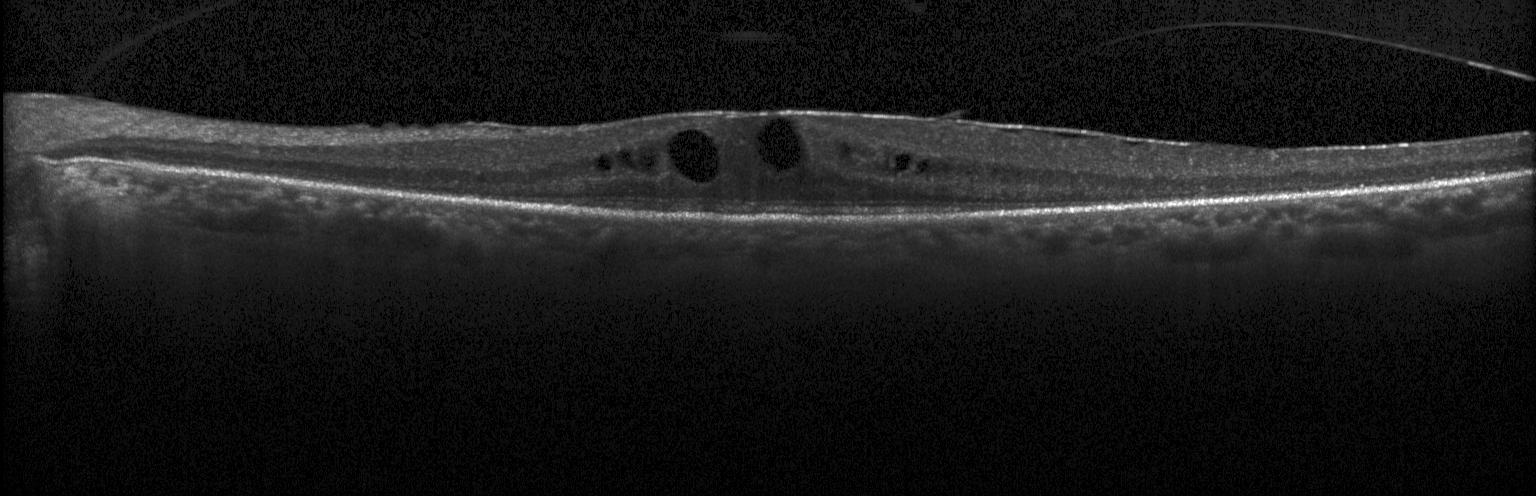
Spectral-domain OCT B-scan: diabetic macular edema.